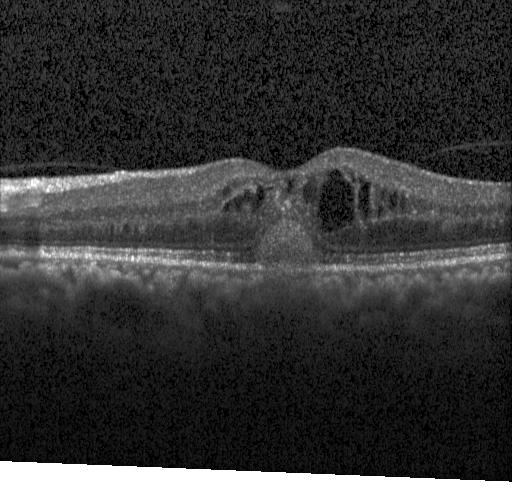
OCT B-scan showing a choroidal neovascular membrane.